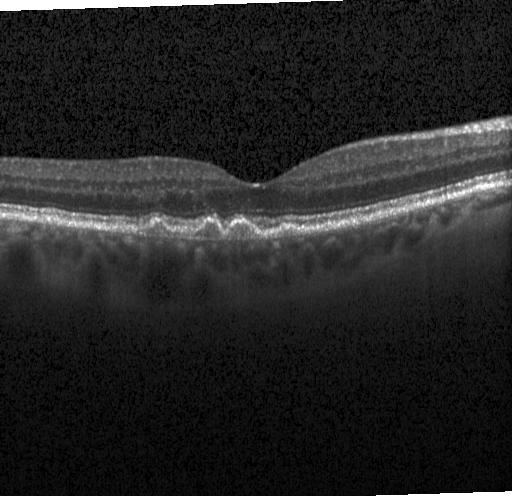 Optical coherence tomography scan — Finding: multiple drusen.